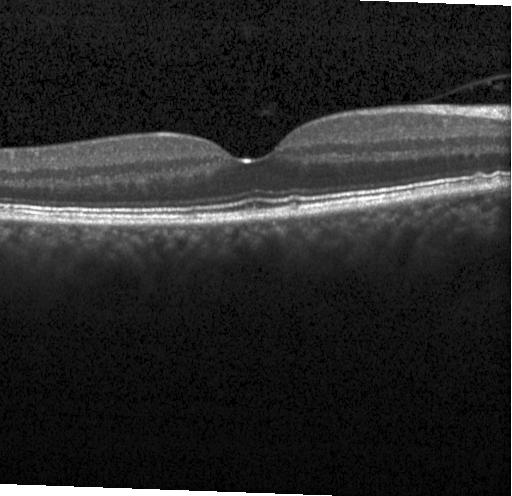

Assessment: no CNV, DME, or drusen.